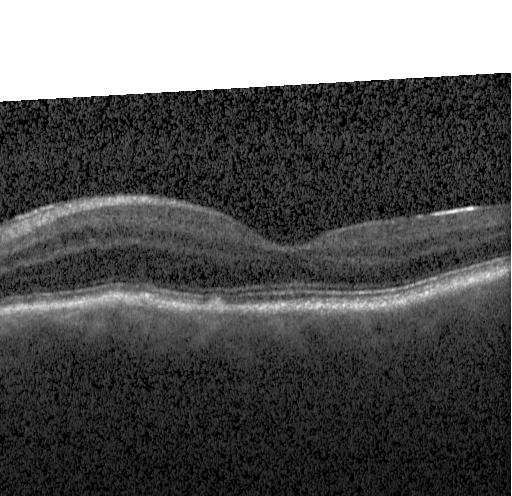

Retinal OCT cross-section — Multiple drusen.